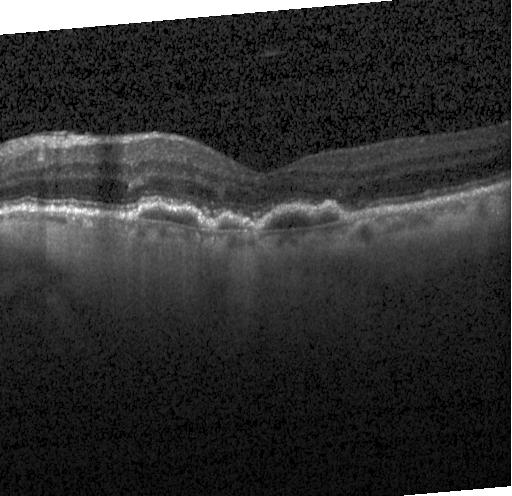

OCT B-scan. Heidelberg Spectralis. Spectral-domain OCT. Horizontal scan through the fovea — Diagnosis: a choroidal neovascular membrane.